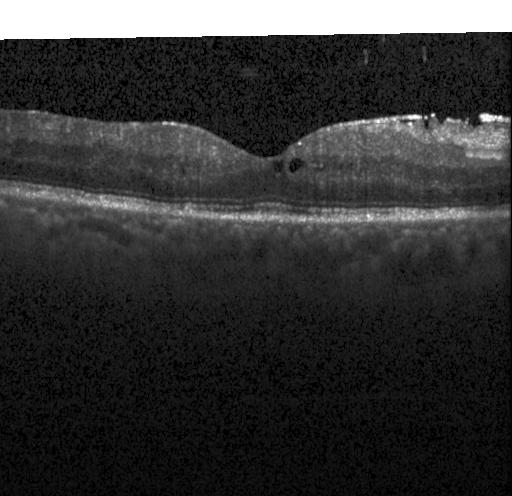
Finding: DME.